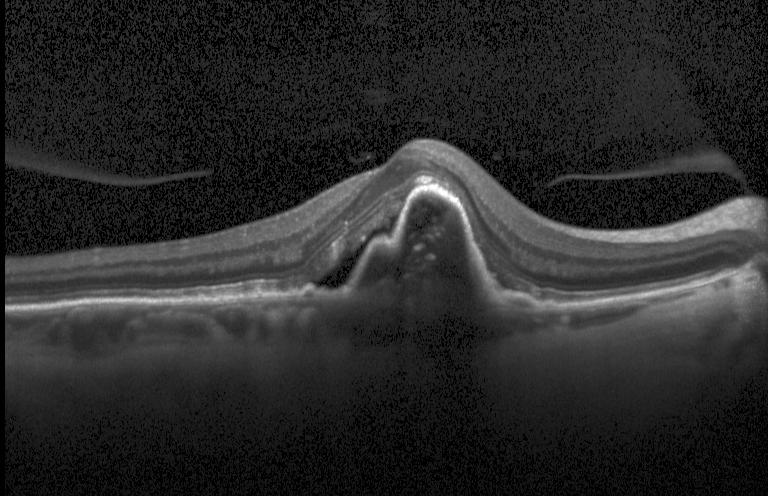
Impression: a choroidal neovascular membrane.